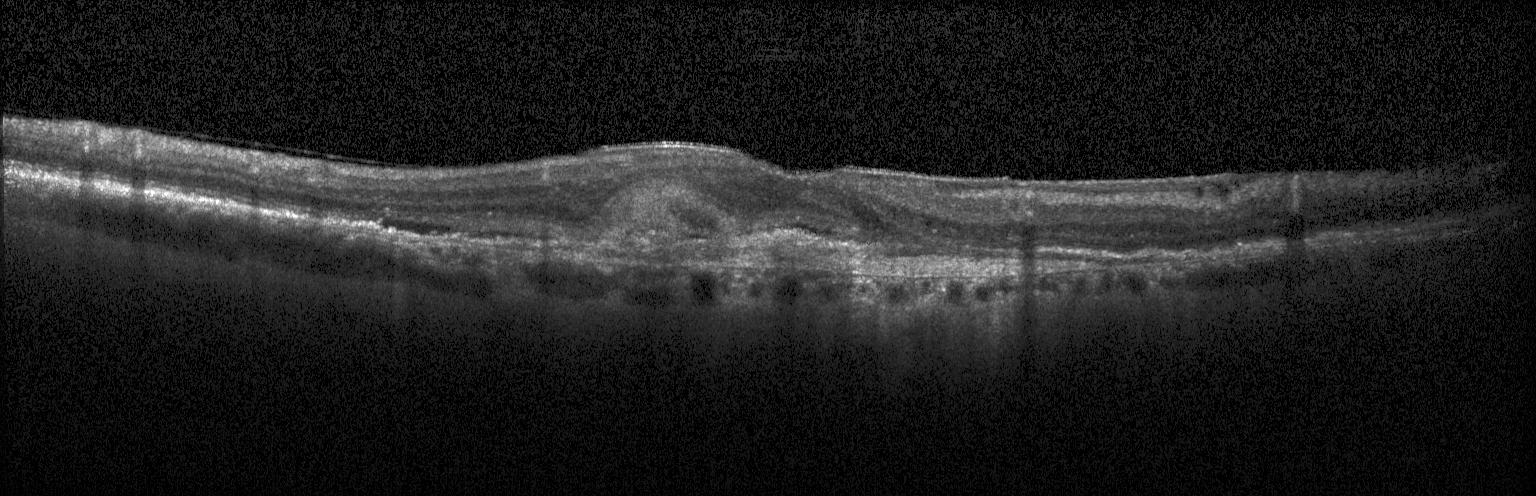
Retinal OCT cross-section.
Diagnosis: choroidal neovascularization.